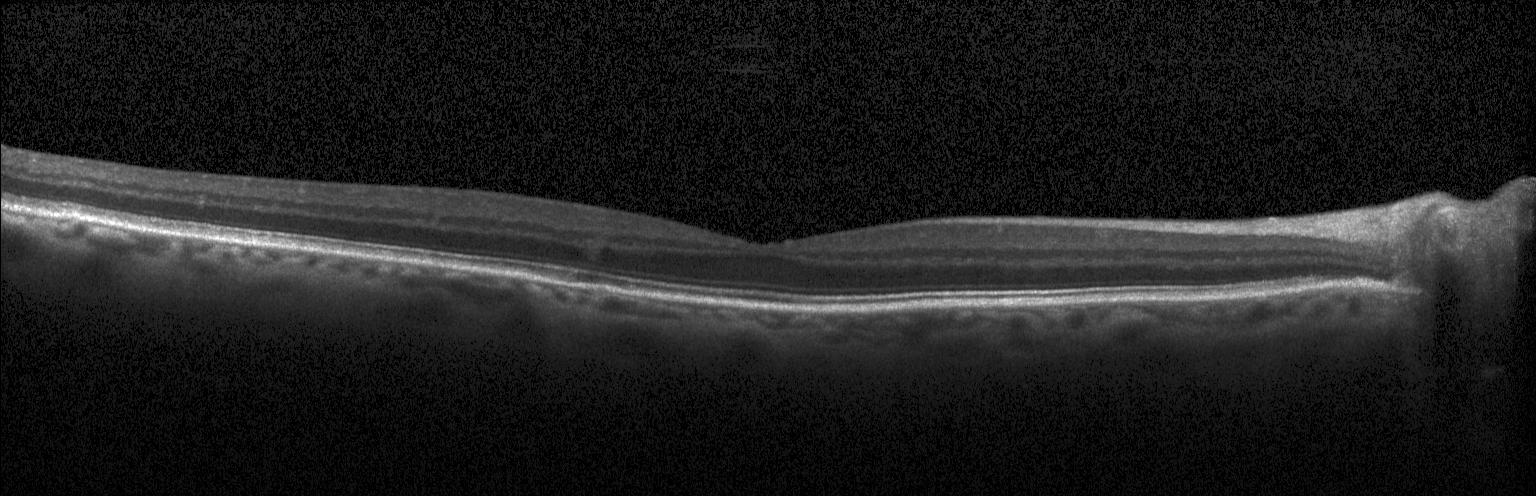

Retinal OCT B-scan · Heidelberg Spectralis · fovea-centered.
Finding: neither CNV, DME, nor drusen.